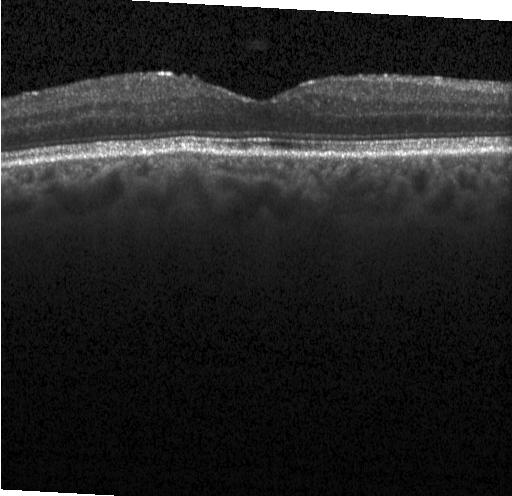

Finding: neither choroidal neovascularization, diabetic macular edema, nor drusen.